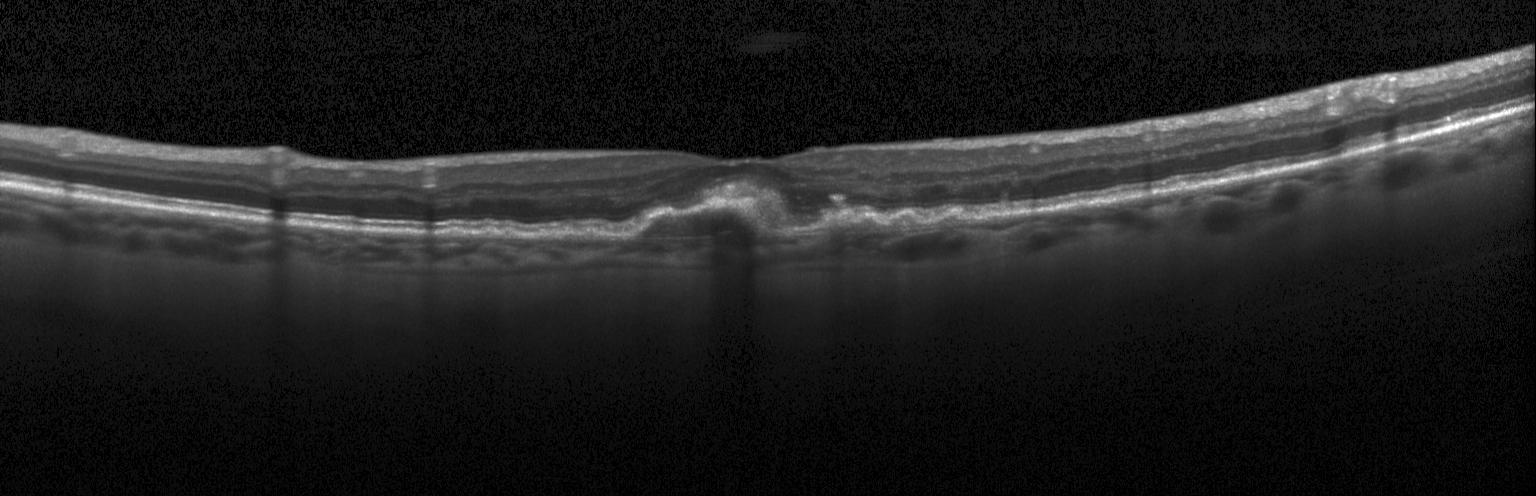
Optical coherence tomography scan; spectral-domain OCT.
This B-scan demonstrates a choroidal neovascular membrane.